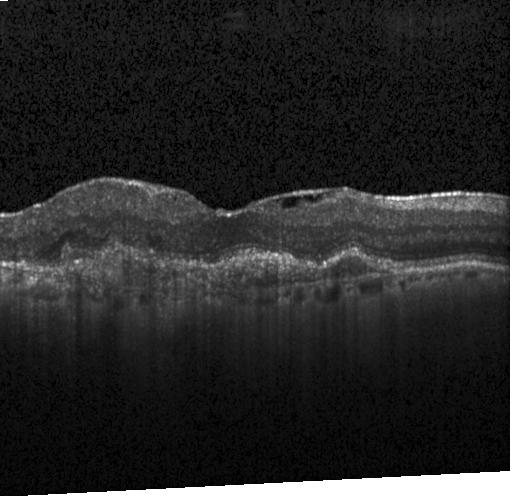
Horizontal scan through the fovea, acquired on a Heidelberg Spectralis, optical coherence tomography B-scan, spectral-domain OCT. Impression: CNV.